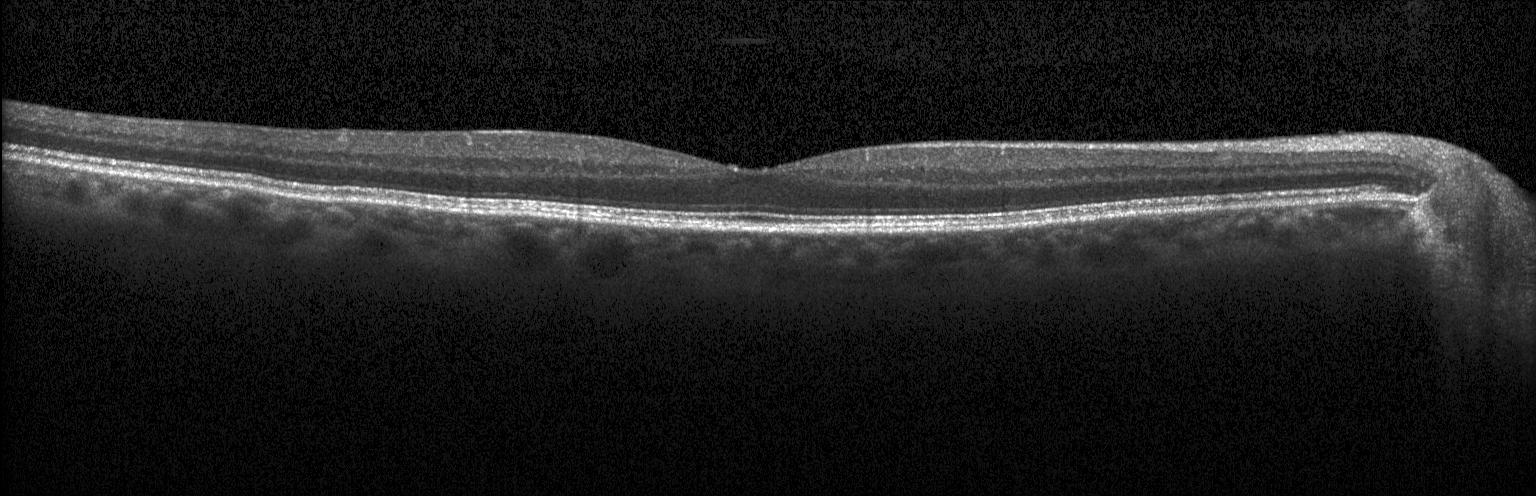

Optical coherence tomography B-scan · Heidelberg Spectralis. The scan shows no evidence of CNV, DME, or drusen.